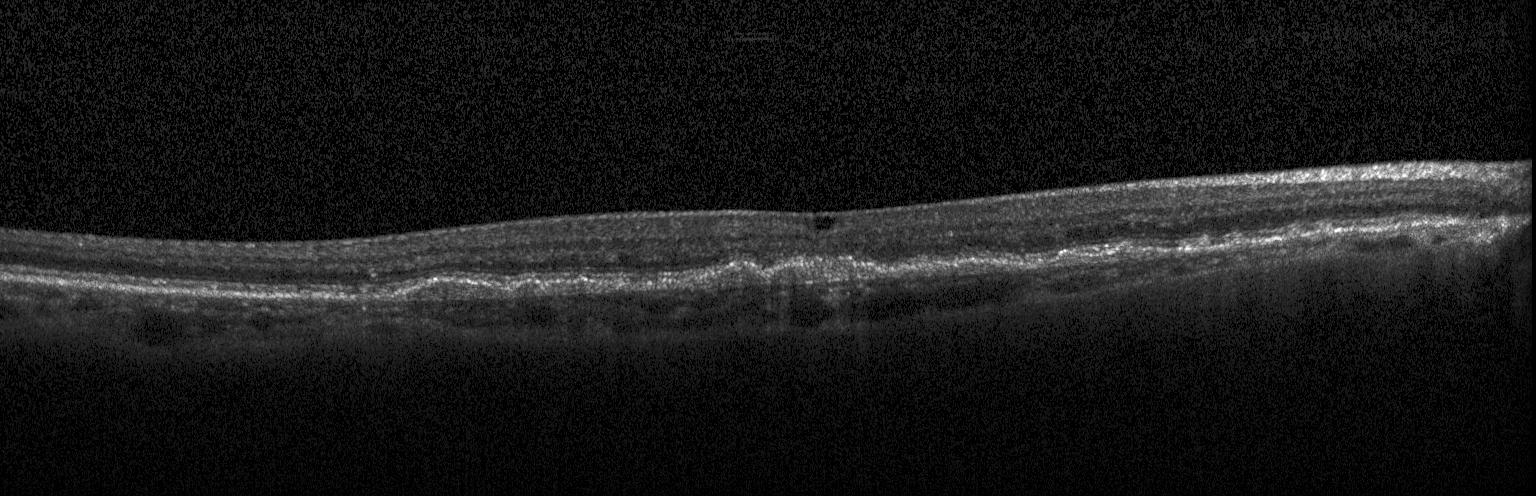 Heidelberg Spectralis; OCT line scan; centered on the fovea — Diagnosis: choroidal neovascularization (CNV).